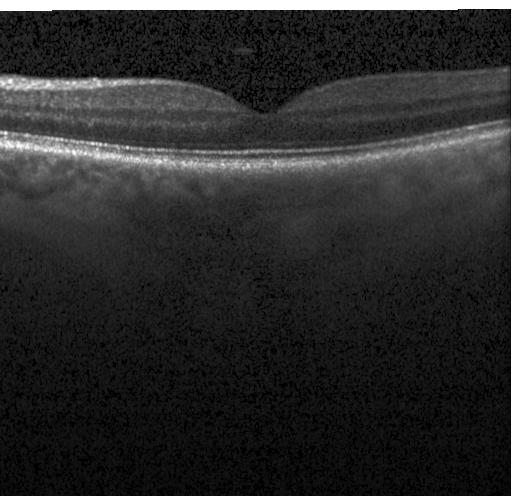
OCT B-scan. Finding: no choroidal neovascularization, no diabetic macular edema, and no drusen.